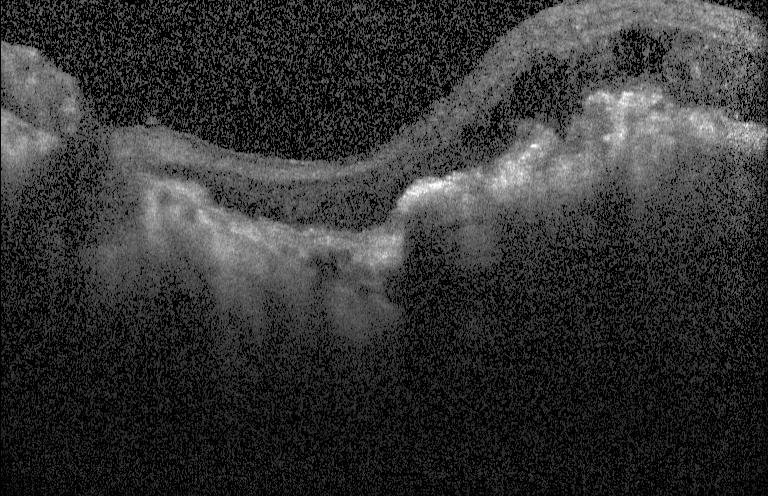

Spectral-domain optical coherence tomography; acquired on a Heidelberg Spectralis; through the macula; OCT line scan. Impression: CNV.